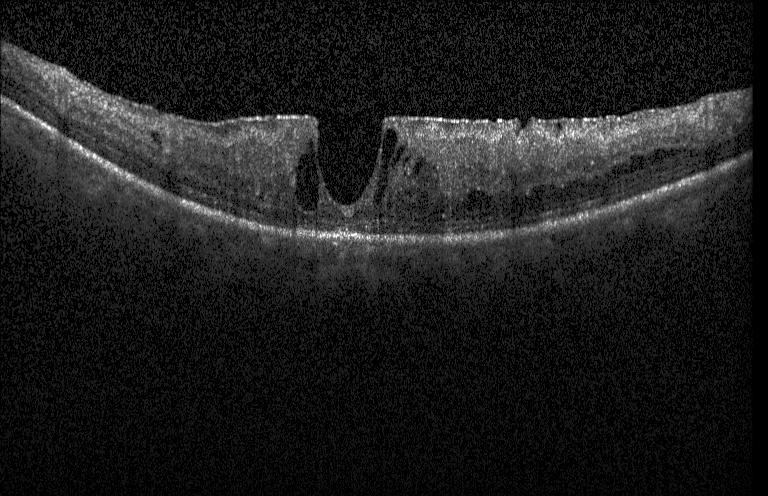
The scan shows diabetic macular edema (DME).